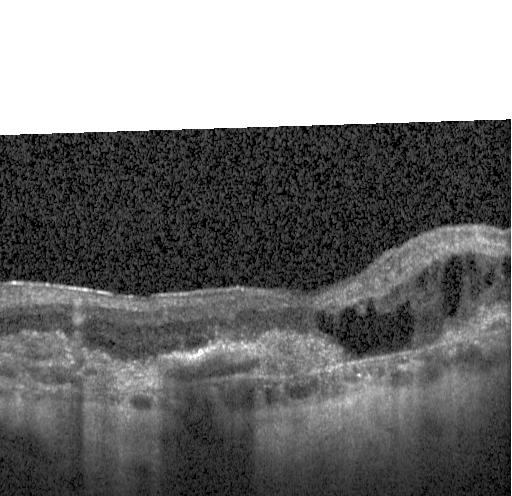

Dx: a choroidal neovascular membrane.